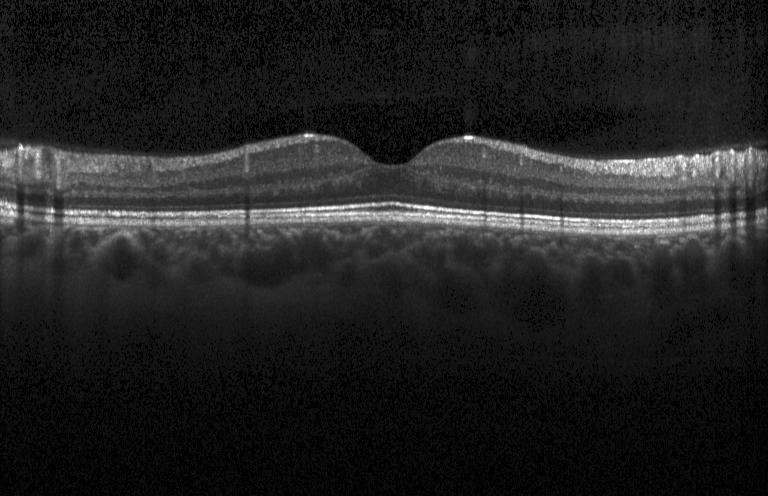

Heidelberg Spectralis OCT system · optical coherence tomography scan — Finding: no CNV, DME, or drusen.